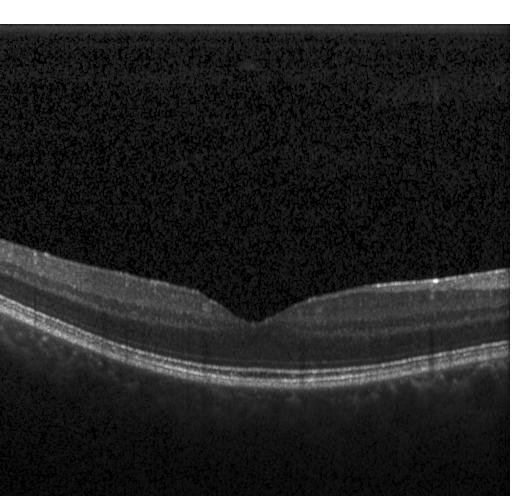
No evidence of CNV, DME, or drusen.